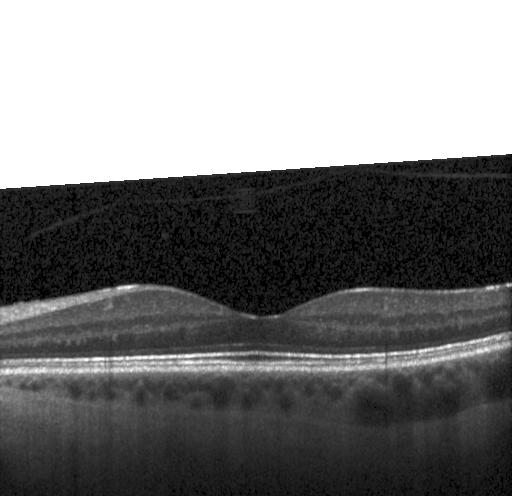
Optical coherence tomography B-scan; through the macula; Heidelberg Spectralis
Impression: no choroidal neovascularization, diabetic macular edema, or drusen.